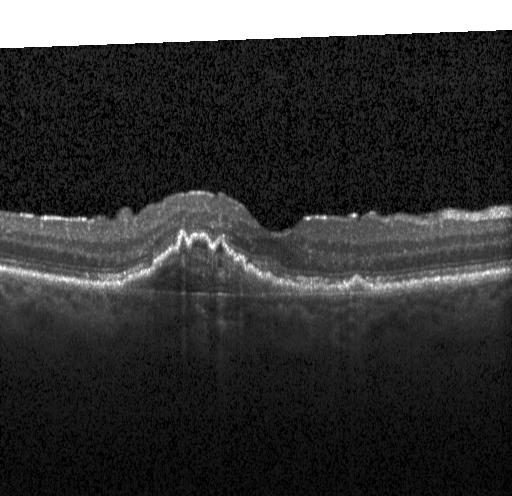

Spectral-domain OCT · OCT line scan · horizontal scan through the fovea
Diagnosis: a choroidal neovascular membrane.